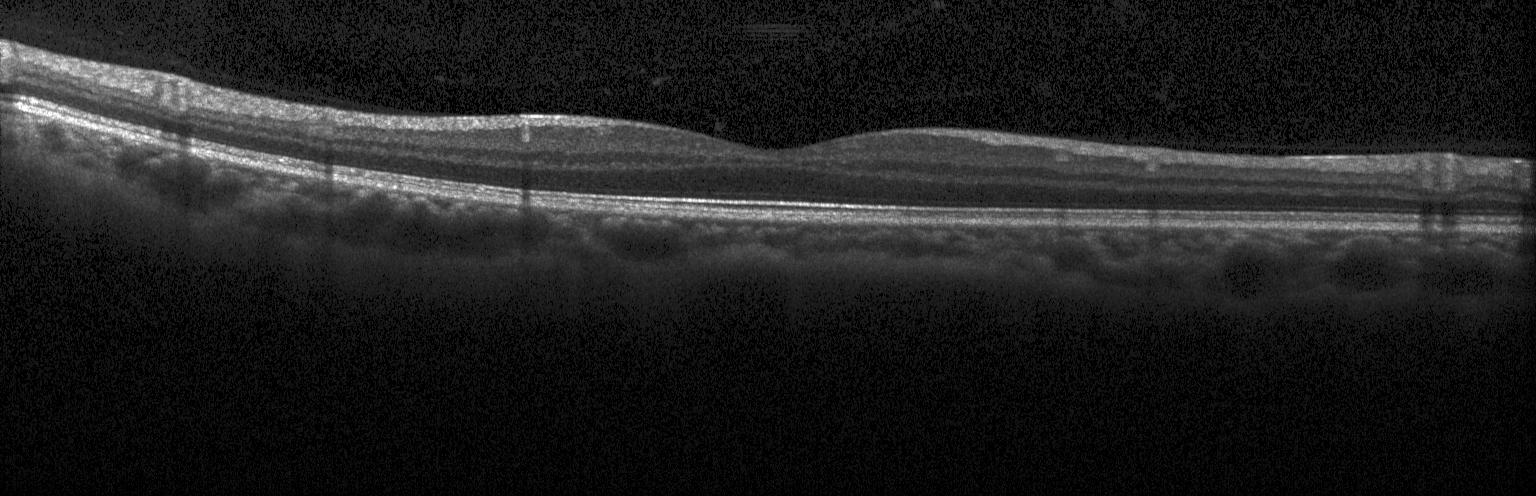
OCT B-scan
Dx: no evidence of choroidal neovascularization, diabetic macular edema, or drusen.